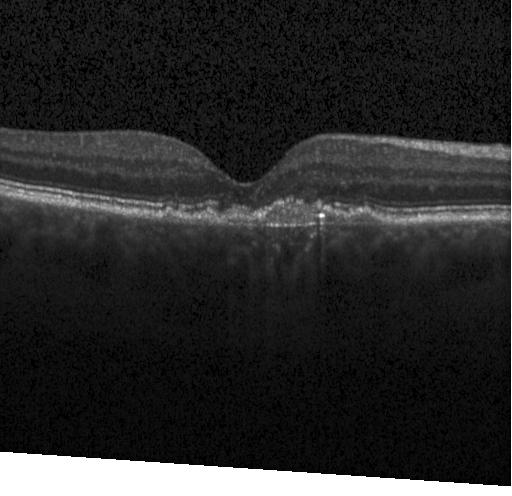 OCT line scan — The scan shows a choroidal neovascular membrane.